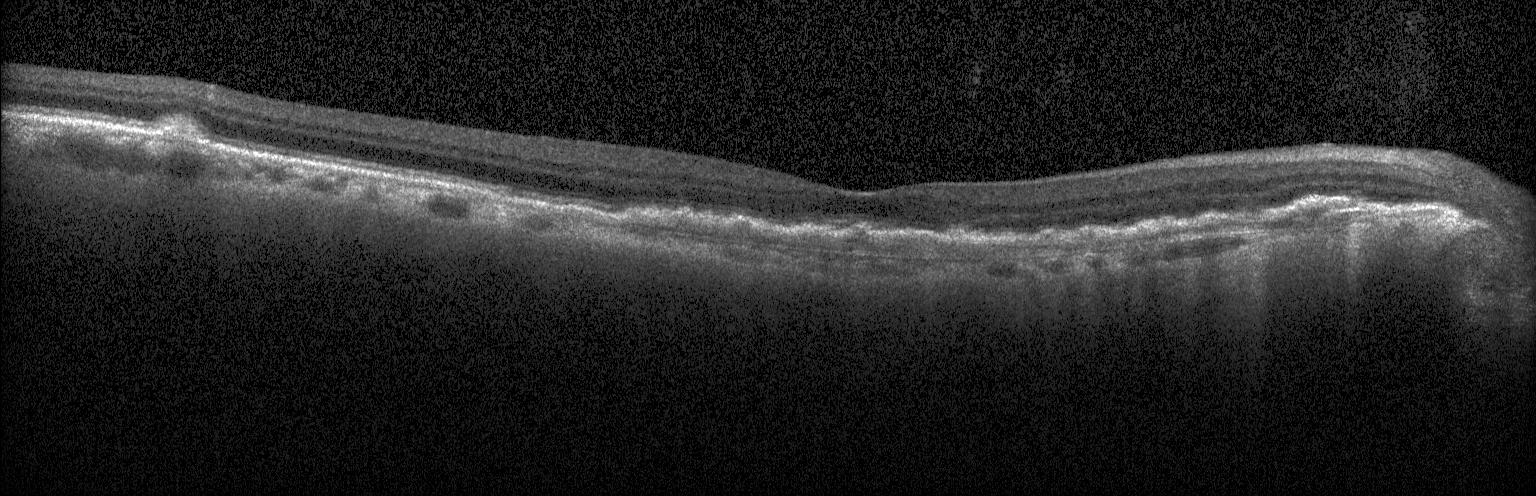
Finding: a choroidal neovascular membrane.